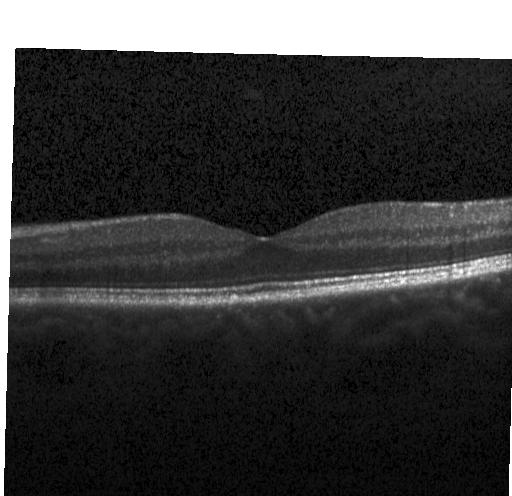
Macular OCT: no evidence of CNV, DME, or drusen.